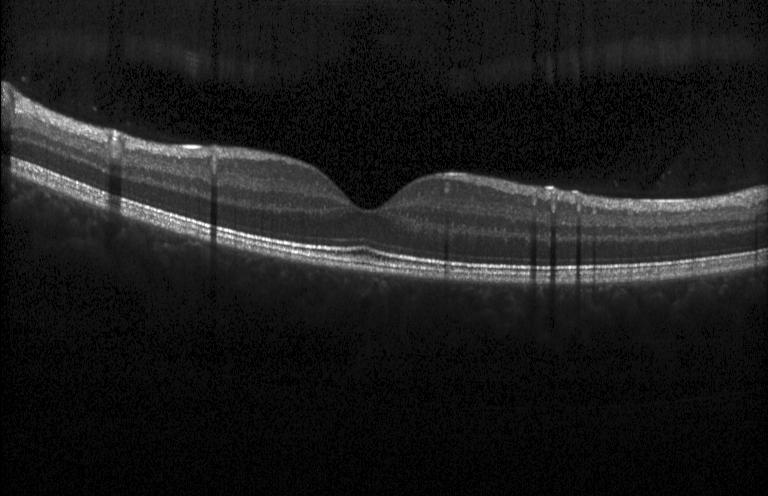
Macular OCT: no CNV, DME, or drusen.